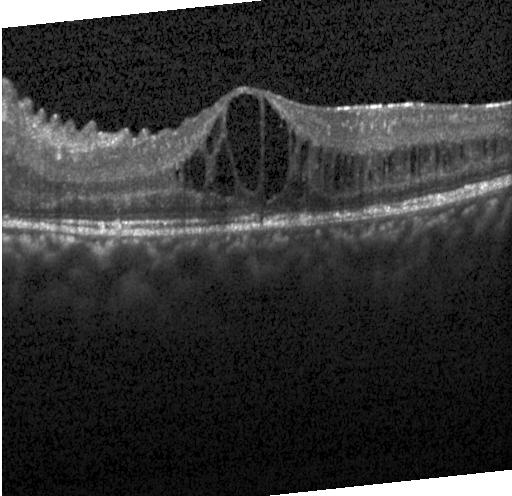
Centered on the fovea. OCT line scan. Instrument: Heidelberg Spectralis. Spectral-domain OCT. Diagnosis: diabetic macular edema.